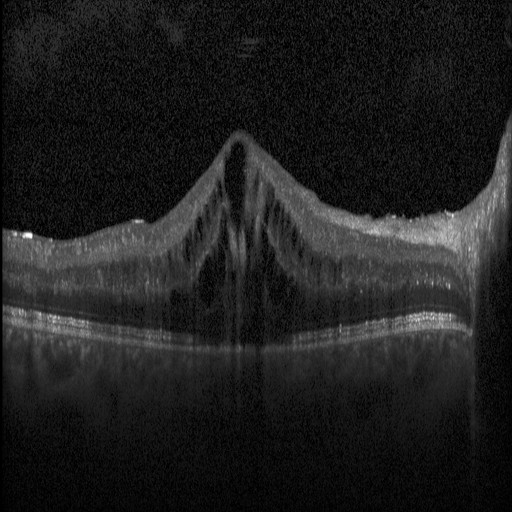 Instrument: Heidelberg Spectralis. SD-OCT. Optical coherence tomography scan
Finding: DME.